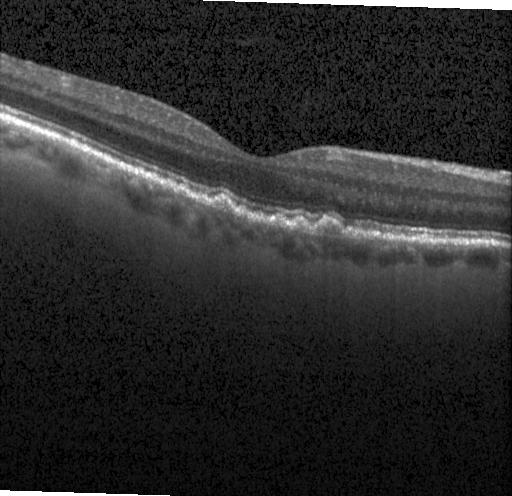 Spectral-domain OCT B-scan: multiple drusen.